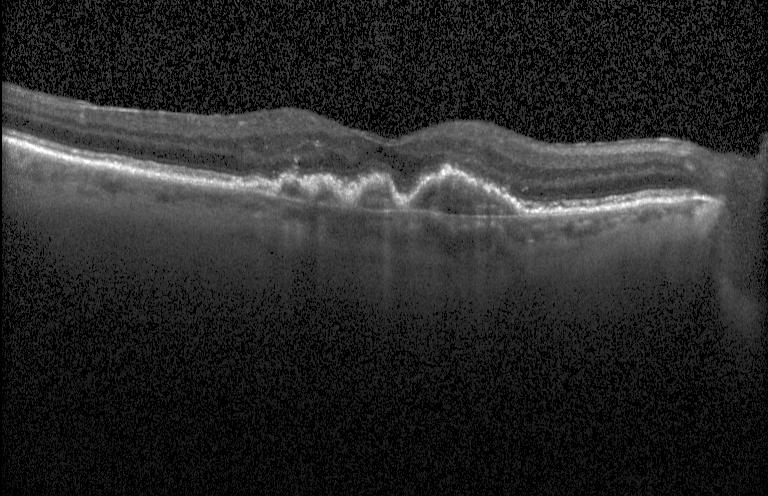

SD-OCT, retinal OCT cross-section, horizontal scan through the fovea, Heidelberg Spectralis OCT system. Finding: a choroidal neovascular membrane.